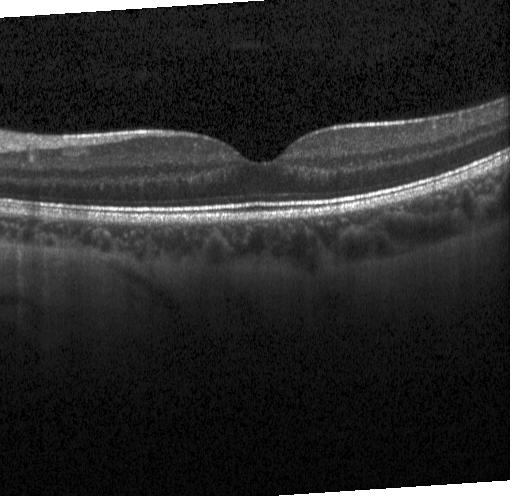
OCT scan showing neither CNV, DME, nor drusen.